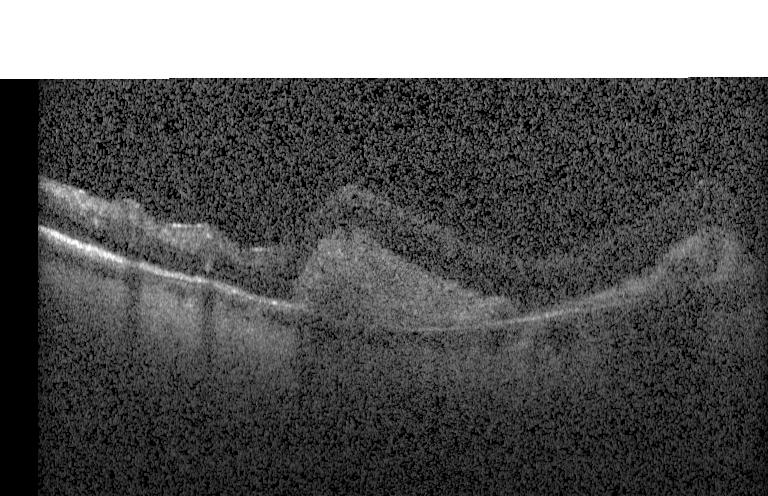 Instrument: Heidelberg Spectralis; OCT B-scan; centered on the fovea — Macular OCT: a choroidal neovascular membrane.